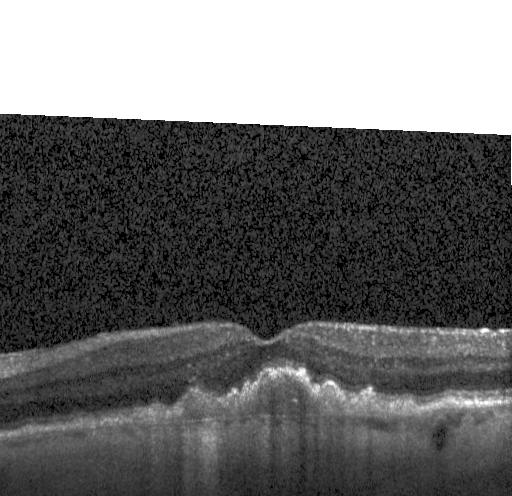
Optical coherence tomography B-scan. Through the macula. Spectral-domain optical coherence tomography. Heidelberg Spectralis OCT system.
Impression: a choroidal neovascular membrane.